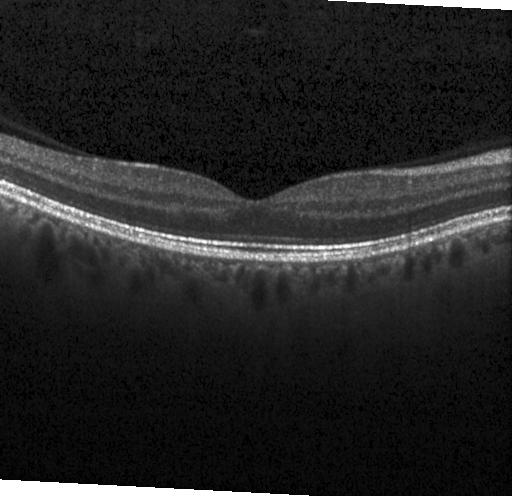
This B-scan demonstrates no evidence of choroidal neovascularization, diabetic macular edema, or drusen.